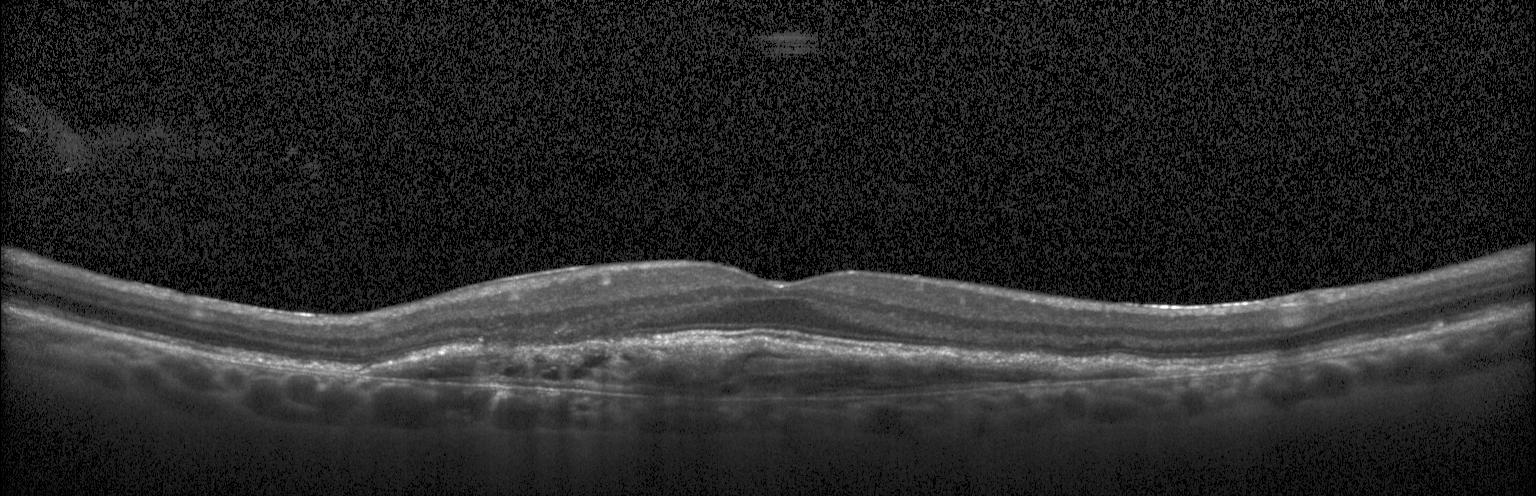
Heidelberg Spectralis, SD-OCT, retinal OCT cross-section
The scan shows a choroidal neovascular membrane.